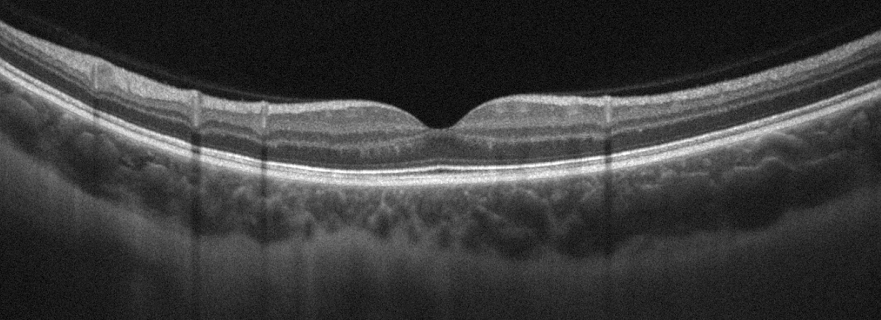 Through the macula; OCT line scan. No evidence of AMD, DME, ERM, RAO, RVO, or VID.